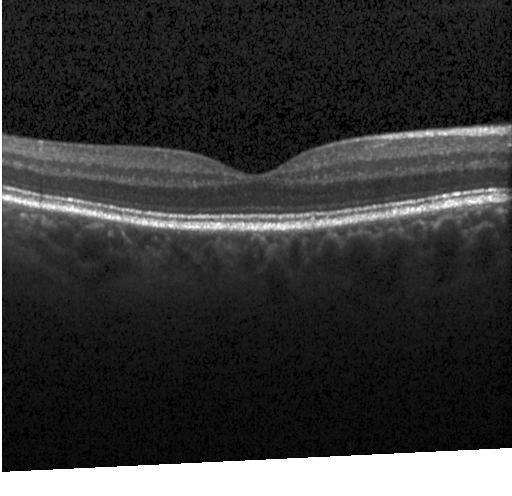
Spectral-domain optical coherence tomography, OCT line scan — Dx: no choroidal neovascularization, diabetic macular edema, or drusen.